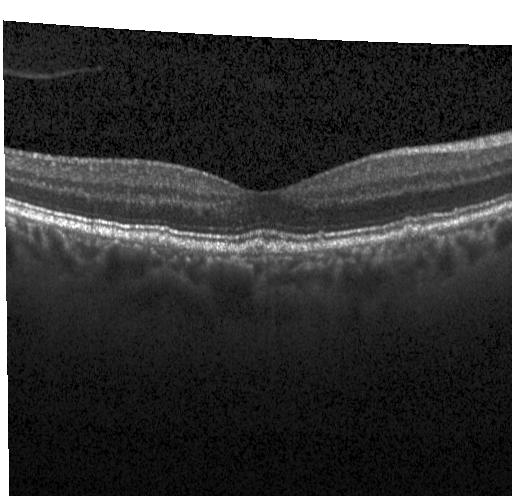 Impression: multiple drusen.